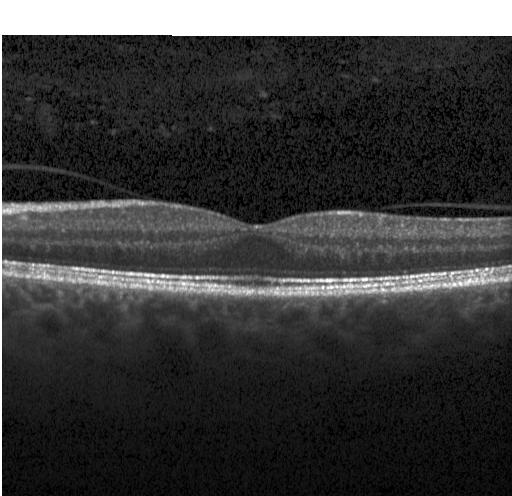

Heidelberg Spectralis OCT system · through the macula · optical coherence tomography B-scan. Diagnosis: no choroidal neovascularization, diabetic macular edema, or drusen.